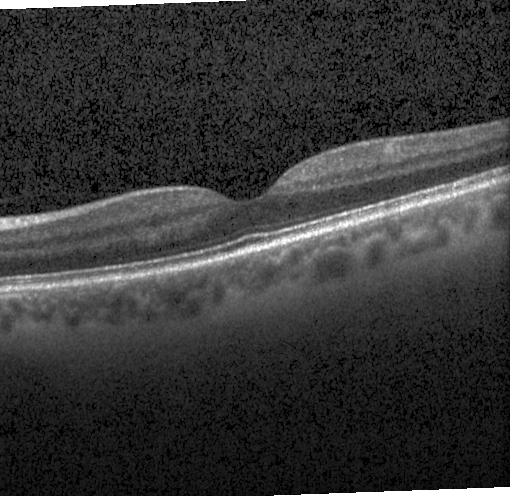

Acquired on a Heidelberg Spectralis; OCT B-scan; macular scan; SD-OCT — Assessment: neither choroidal neovascularization, diabetic macular edema, nor drusen.